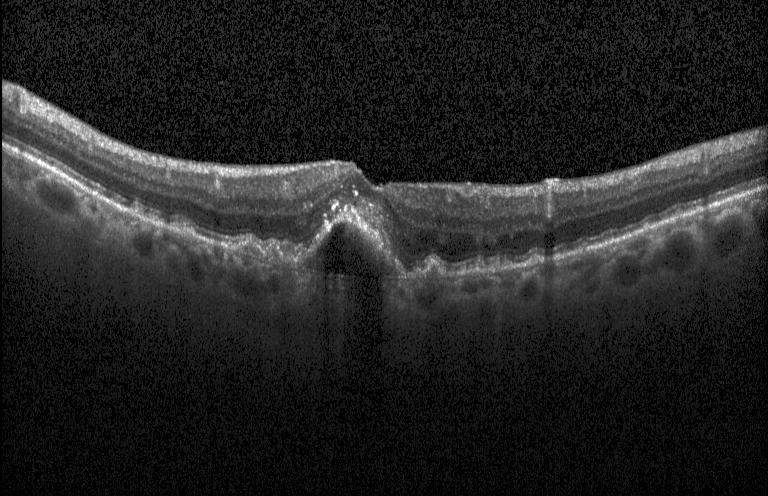 Diagnosis: a choroidal neovascular membrane.